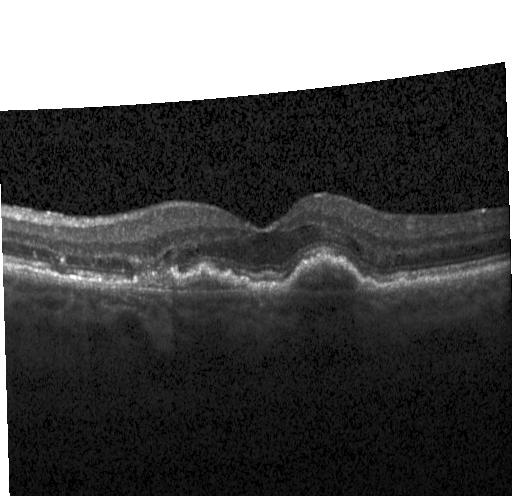
Diagnosis: a choroidal neovascular membrane.